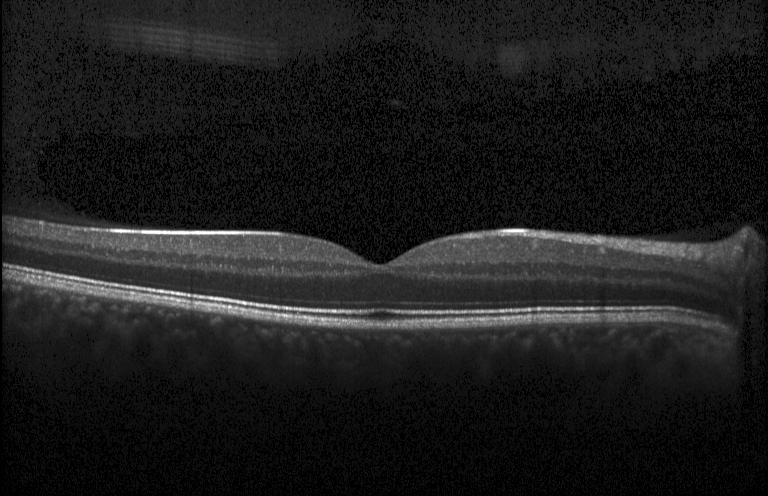
OCT scan showing no evidence of choroidal neovascularization, diabetic macular edema, or drusen.